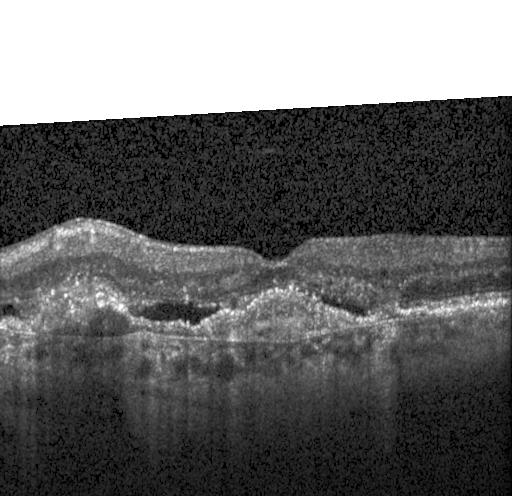
Diagnosis: CNV.